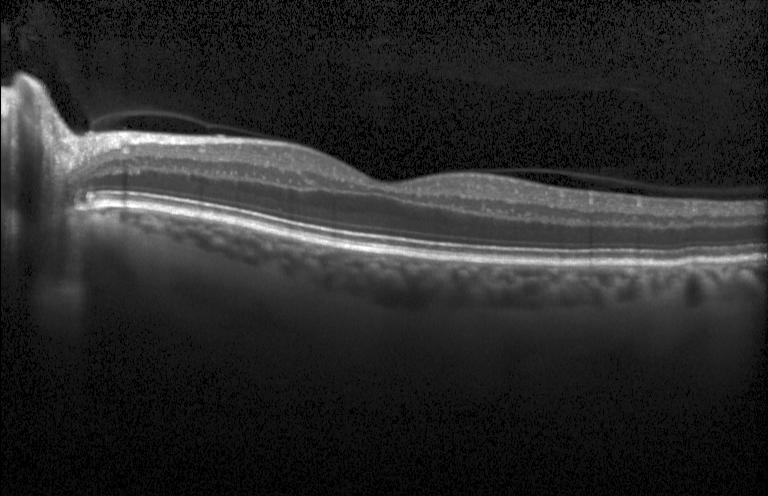

Heidelberg Spectralis. SD-OCT. Horizontal scan through the fovea. Retinal OCT B-scan.
This B-scan demonstrates neither choroidal neovascularization, diabetic macular edema, nor drusen.